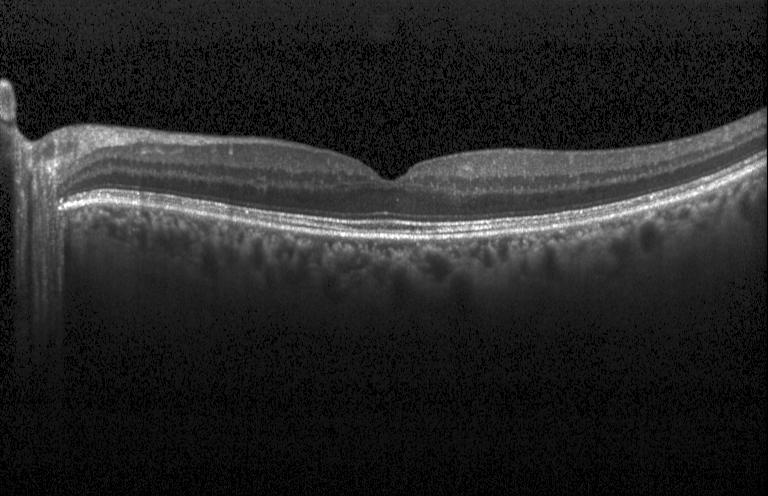

Retinal OCT cross-section, Heidelberg Spectralis, through the macula, SD-OCT
Assessment: neither choroidal neovascularization, diabetic macular edema, nor drusen.